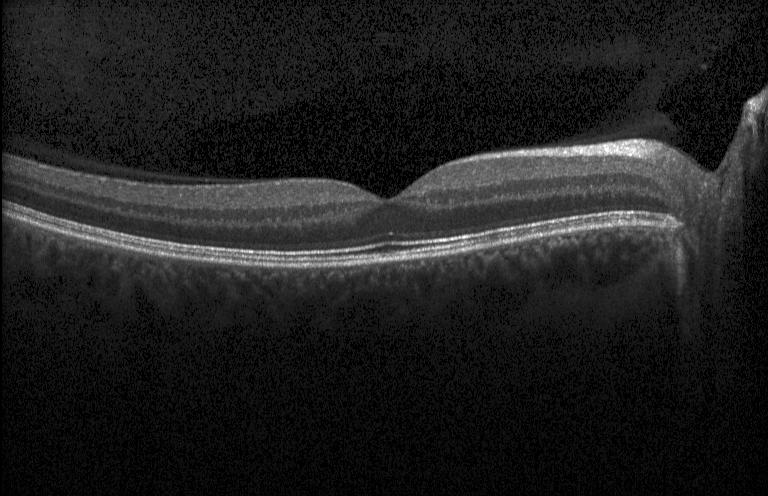 No evidence of choroidal neovascularization, diabetic macular edema, or drusen.